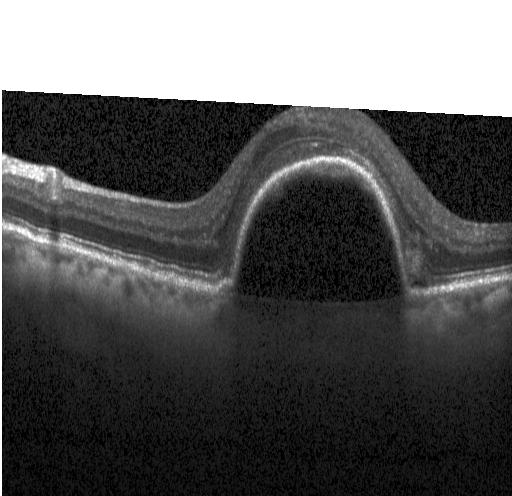

Instrument: Heidelberg Spectralis. Spectral-domain OCT. Retinal OCT B-scan. Macular scan. A choroidal neovascular membrane.